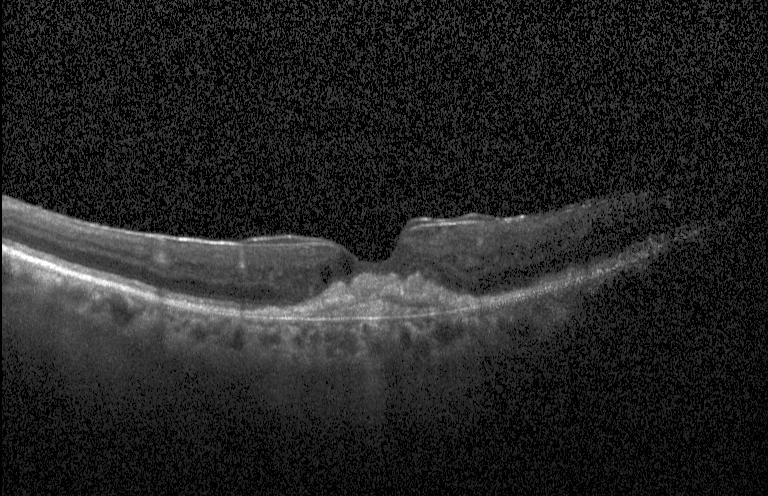

Impression: a choroidal neovascular membrane.